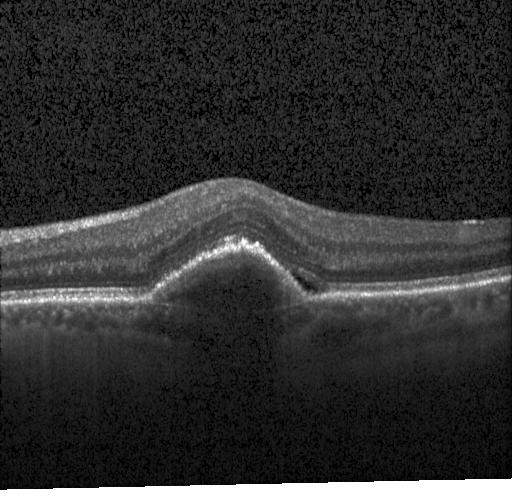
Optical coherence tomography B-scan — Finding: a choroidal neovascular membrane.